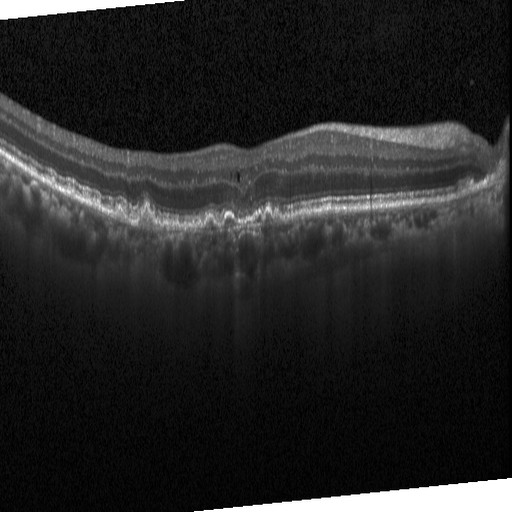
SD-OCT · optical coherence tomography B-scan — Finding: diabetic macular edema (DME).